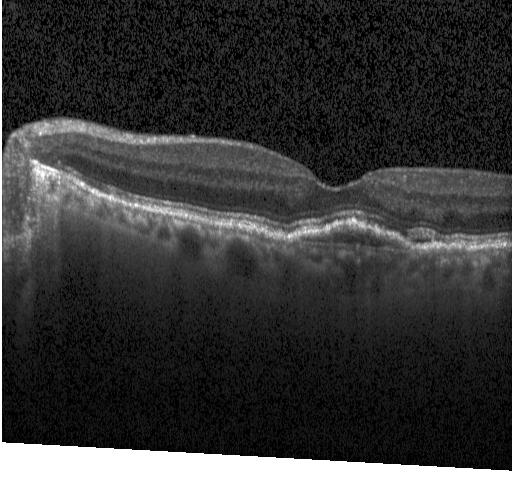 Retinal OCT cross-section showing choroidal neovascularization (CNV).